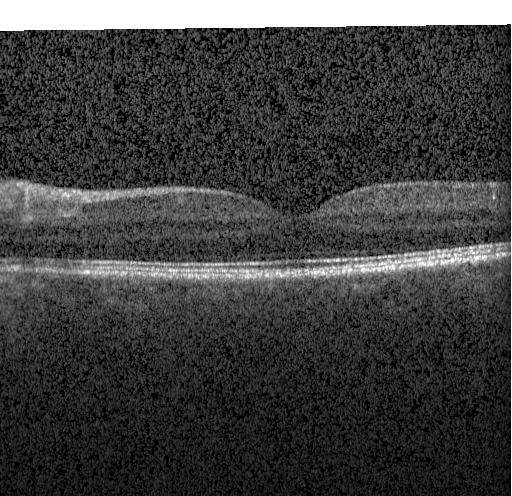

Finding: no CNV, no DME, and no drusen.